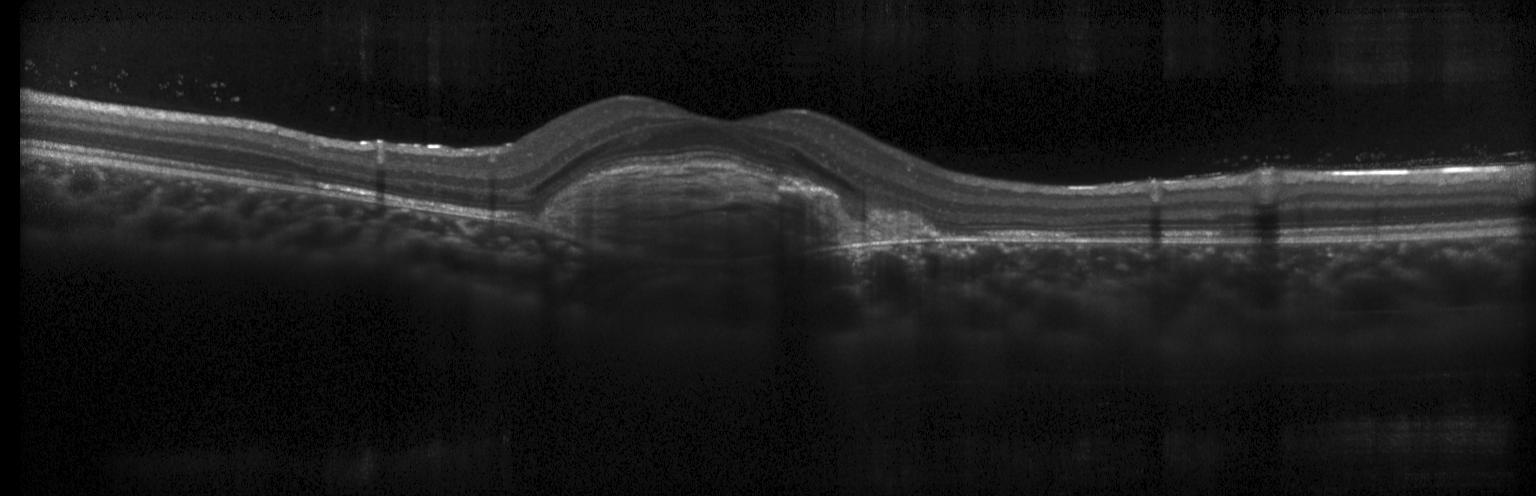 Impression: choroidal neovascularization.